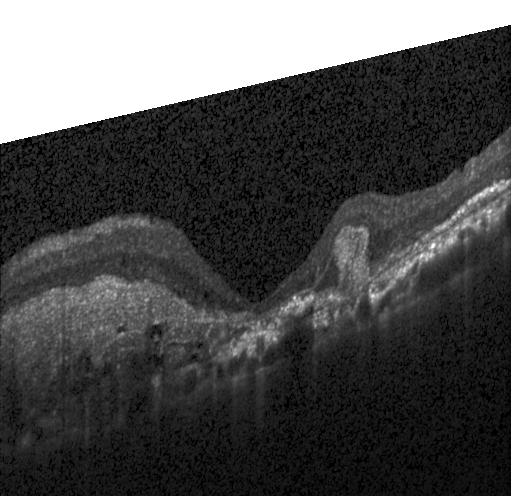 Finding: choroidal neovascularization.